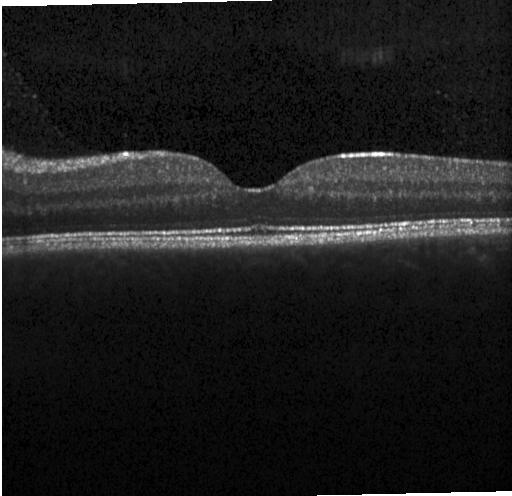
Dx: no choroidal neovascularization, no diabetic macular edema, and no drusen.